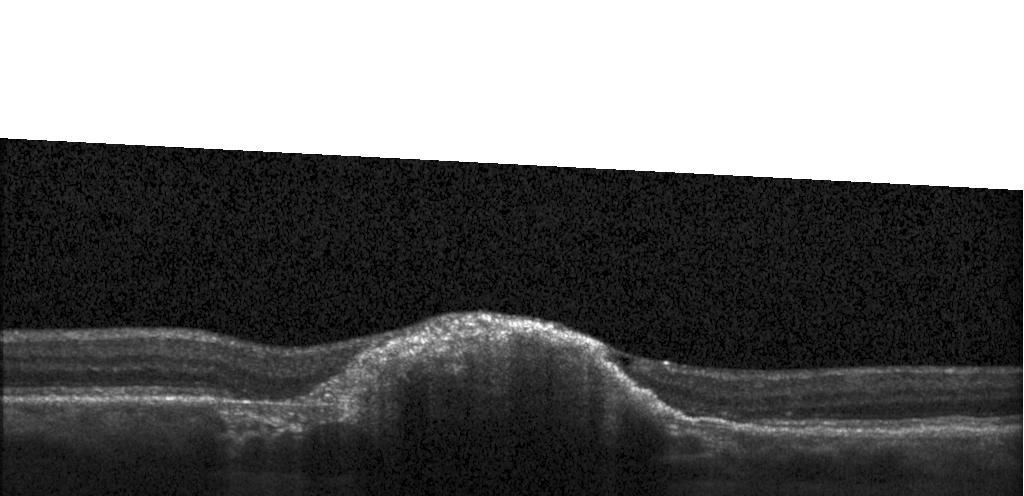
Optical coherence tomography scan — The scan shows choroidal neovascularization.